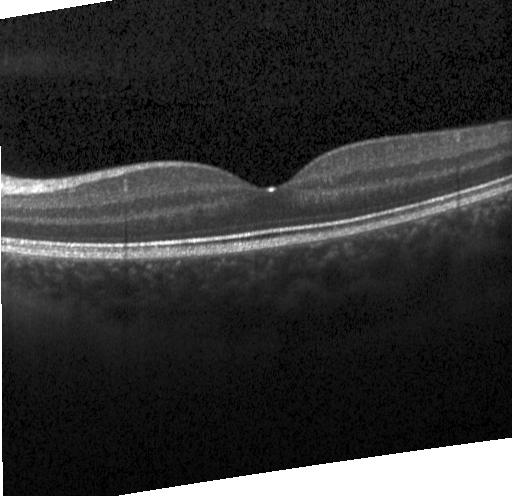
Spectral-domain optical coherence tomography · OCT line scan. The scan shows no evidence of CNV, DME, or drusen.